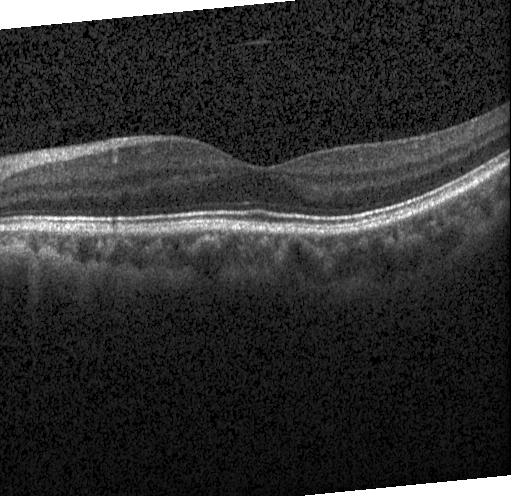
Through the macula, OCT B-scan, acquired on a Heidelberg Spectralis, SD-OCT.
This B-scan demonstrates no evidence of choroidal neovascularization, diabetic macular edema, or drusen.